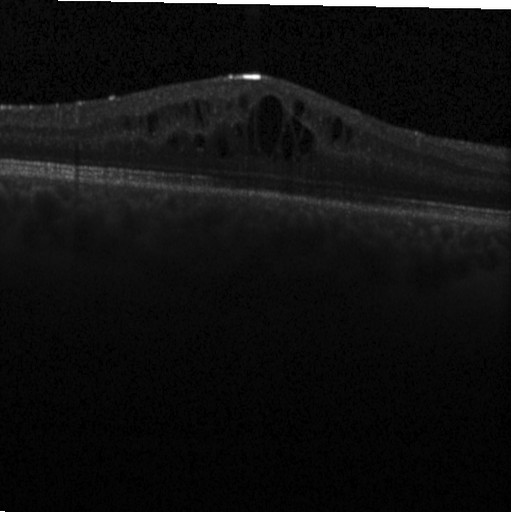

Optical coherence tomography B-scan — Finding: DME.